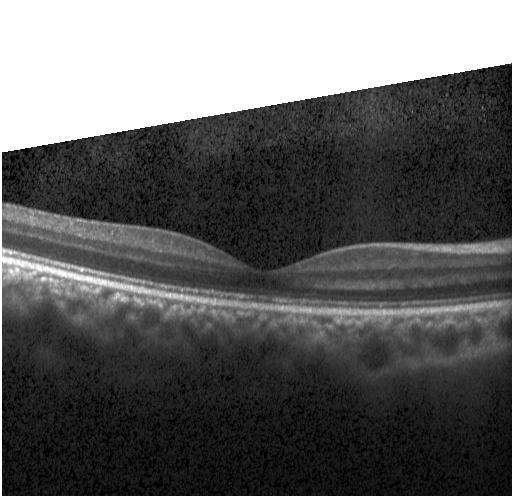

Retinal OCT B-scan. Dx: no choroidal neovascularization, no diabetic macular edema, and no drusen.